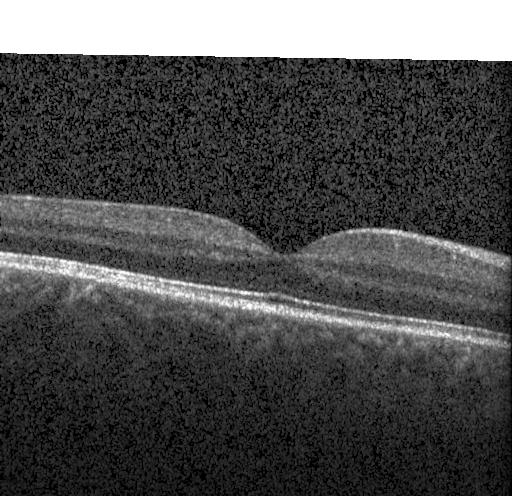
Macular OCT: neither choroidal neovascularization, diabetic macular edema, nor drusen.